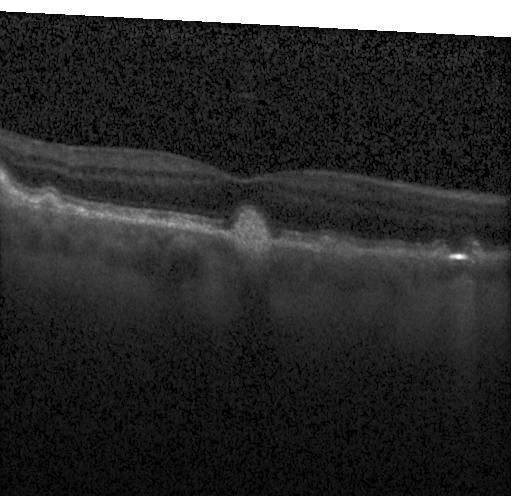 This B-scan demonstrates multiple drusen.